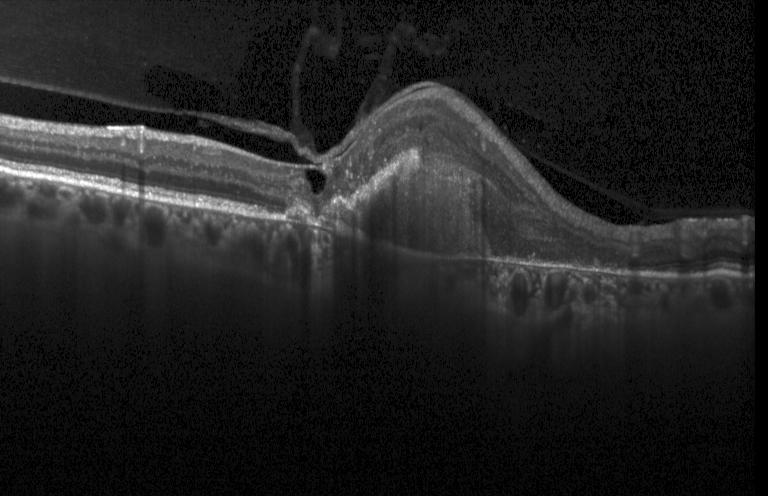

Spectral-domain optical coherence tomography. Centered on the fovea. Optical coherence tomography scan. Acquired on a Heidelberg Spectralis
This B-scan demonstrates a choroidal neovascular membrane.